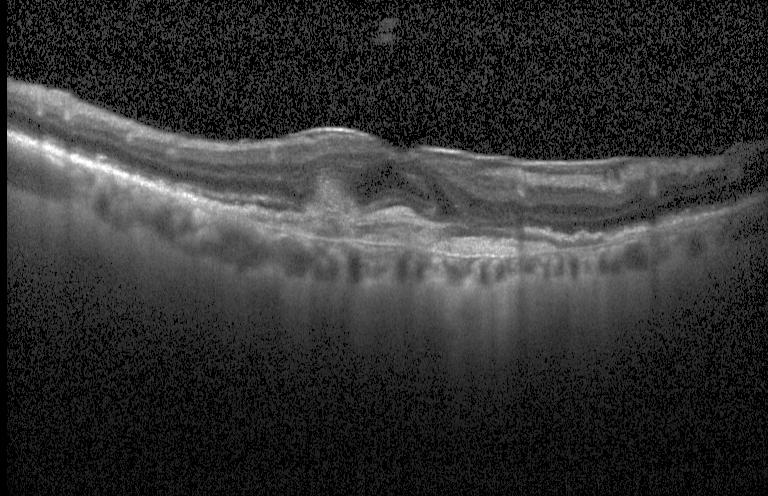

Retinal OCT B-scan · horizontal scan through the fovea · instrument: Heidelberg Spectralis.
Finding: choroidal neovascularization.